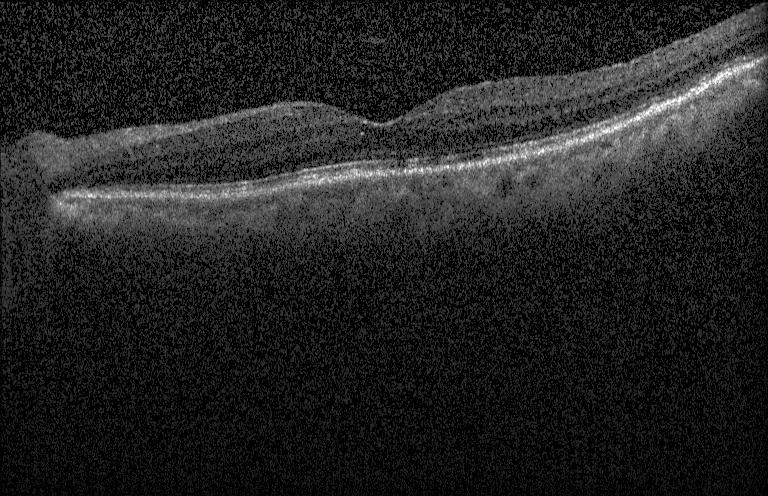

Horizontal scan through the fovea · spectral-domain optical coherence tomography · optical coherence tomography B-scan · acquired on a Heidelberg Spectralis — Impression: no evidence of choroidal neovascularization, diabetic macular edema, or drusen.